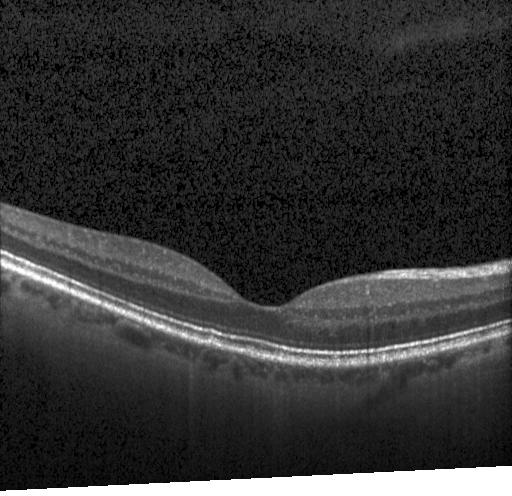
Optical coherence tomography scan; horizontal scan through the fovea; acquired on a Heidelberg Spectralis; spectral-domain OCT.
No choroidal neovascularization, diabetic macular edema, or drusen.